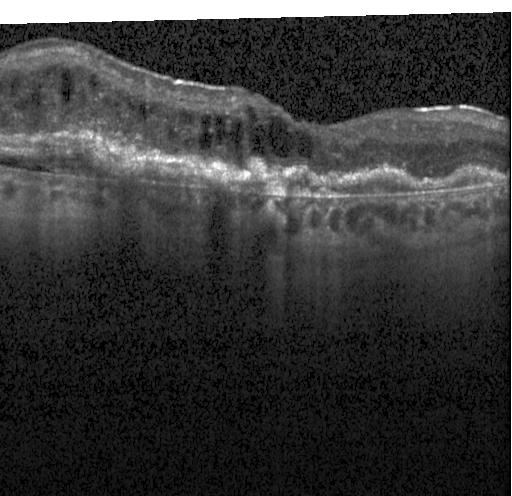

Diagnosis: a choroidal neovascular membrane.